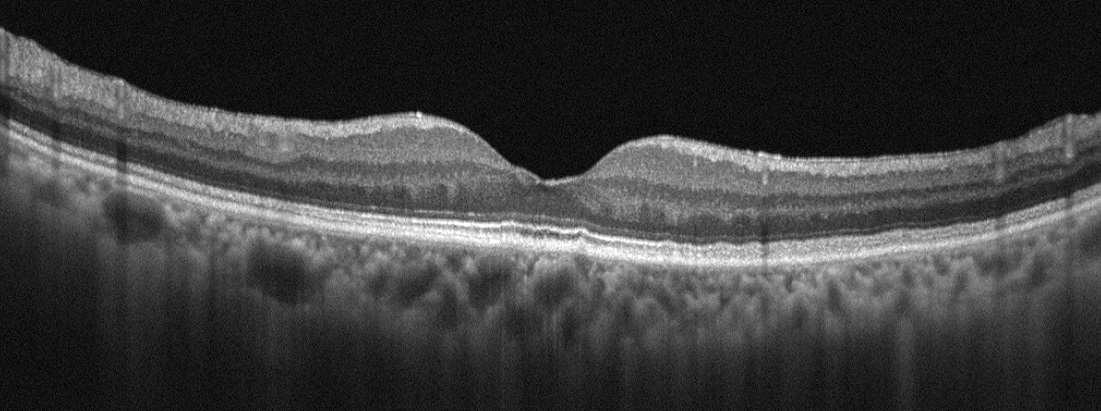

Finding: age-related macular degeneration (AMD).